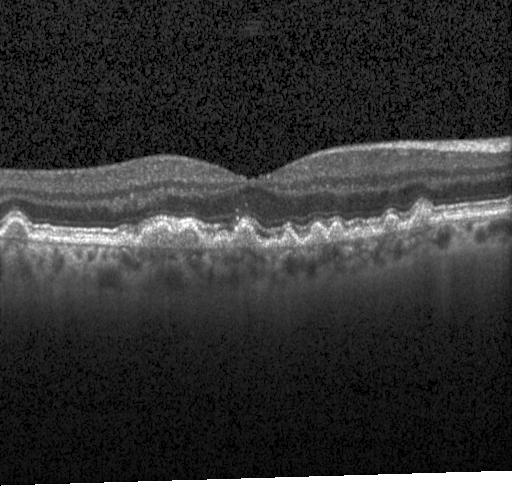 Instrument: Heidelberg Spectralis, retinal OCT cross-section.
Finding: sub-RPE drusenoid deposits.